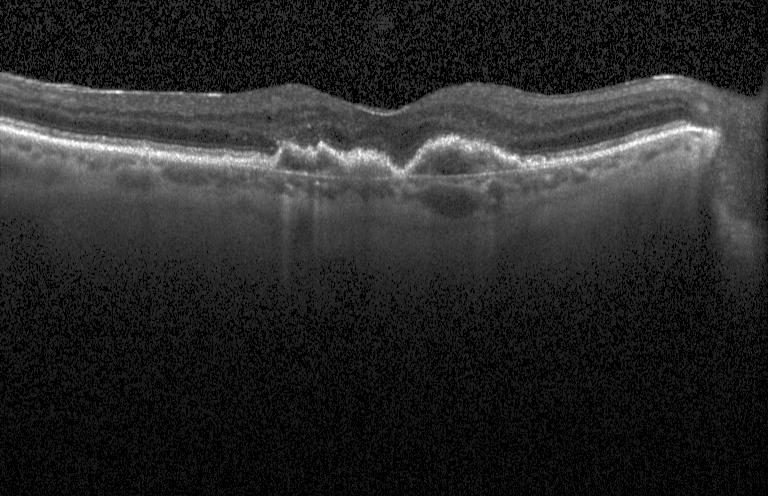 Optical coherence tomography scan; horizontal scan through the fovea; SD-OCT; acquired on a Heidelberg Spectralis
OCT finding: a choroidal neovascular membrane.